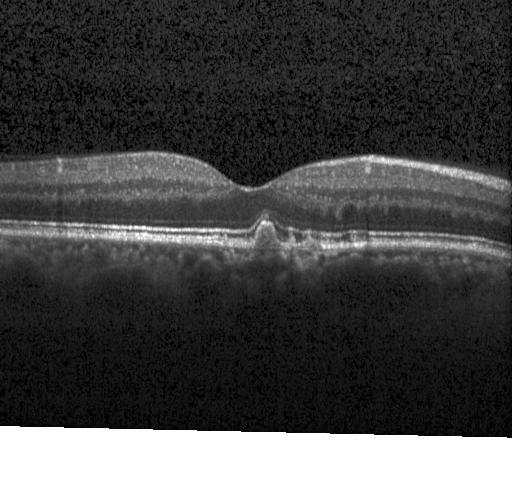 Optical coherence tomography B-scan. Through the macula
OCT finding: sub-RPE drusenoid deposits.